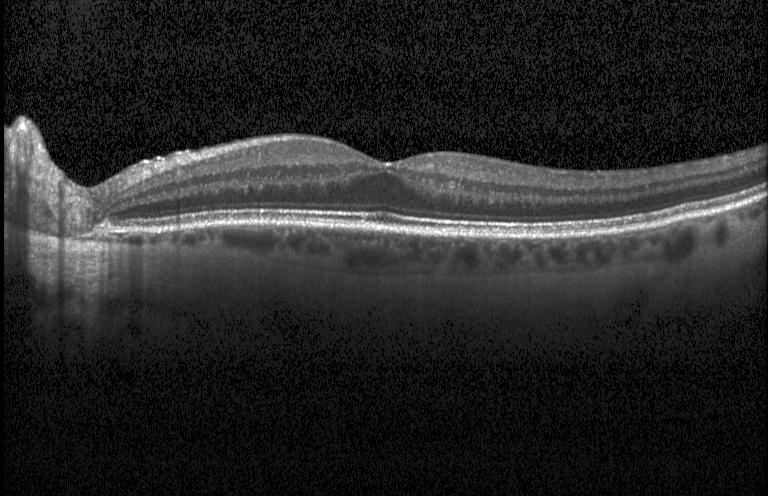
Finding: no CNV, no DME, and no drusen.